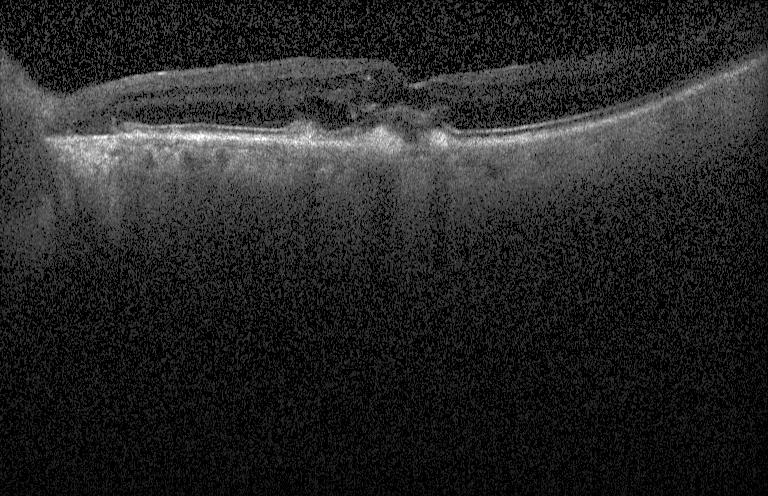
Retinal OCT B-scan. OCT finding: a choroidal neovascular membrane.